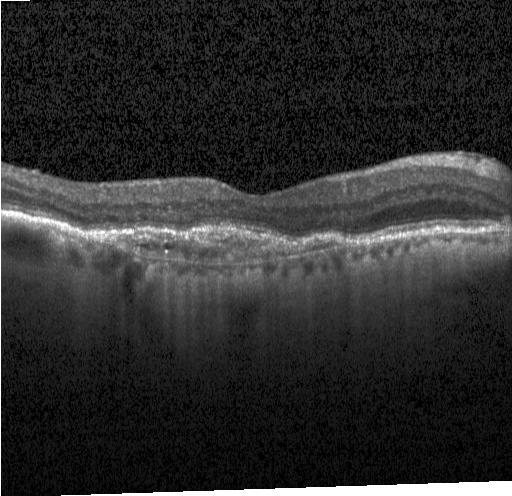

OCT B-scan showing choroidal neovascularization.